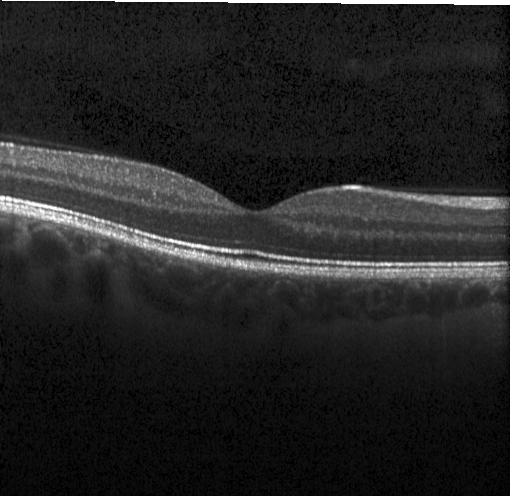 SD-OCT, optical coherence tomography scan, fovea-centered, acquired on a Heidelberg Spectralis. OCT finding: no choroidal neovascularization, no diabetic macular edema, and no drusen.